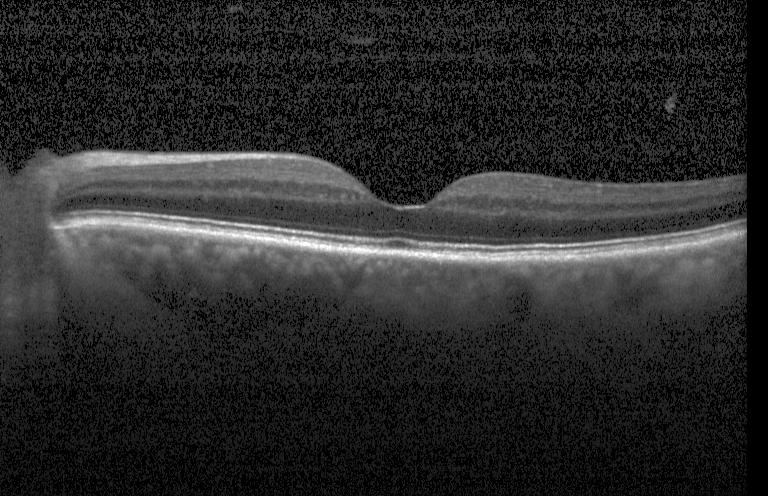
Optical coherence tomography B-scan
Impression: no choroidal neovascularization, no diabetic macular edema, and no drusen.